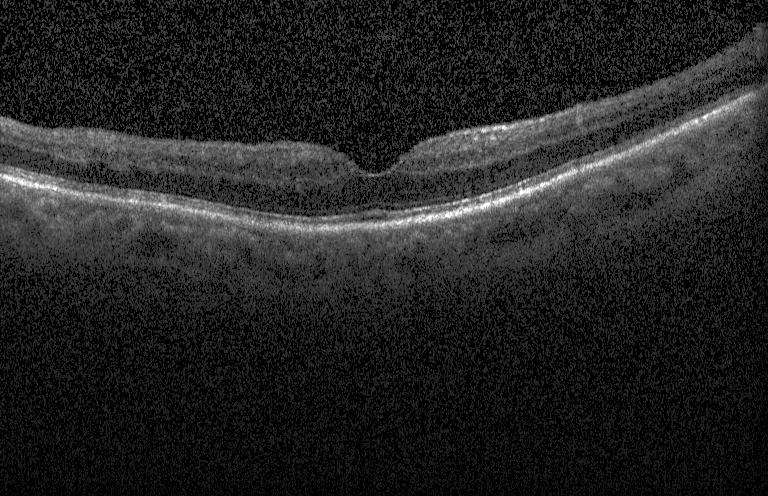 Neither choroidal neovascularization, diabetic macular edema, nor drusen.